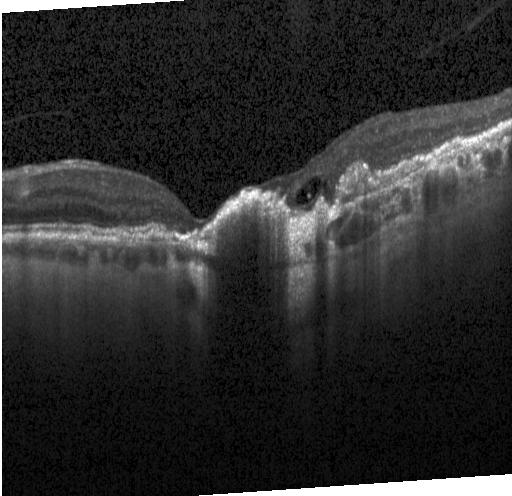 Macular OCT demonstrating CNV.